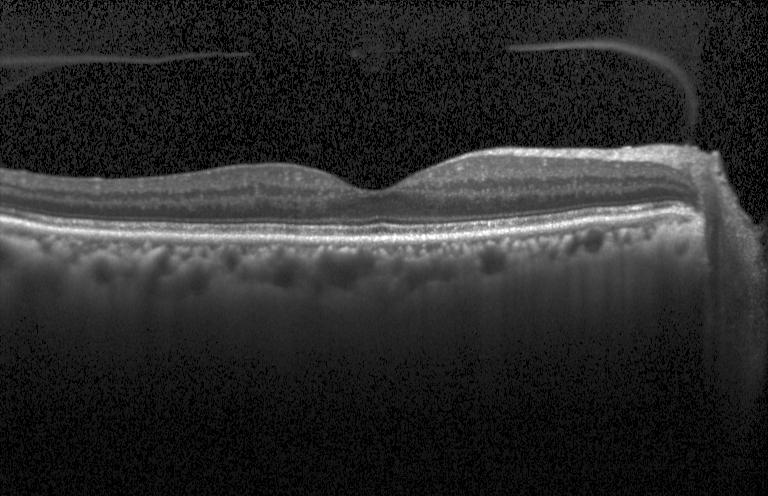
OCT line scan — Impression: no evidence of CNV, DME, or drusen.